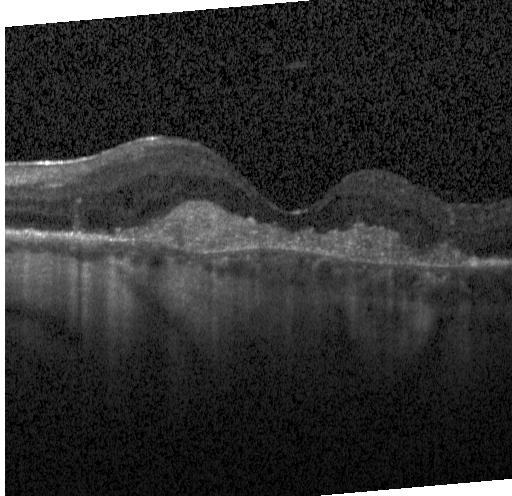
Impression: choroidal neovascularization.